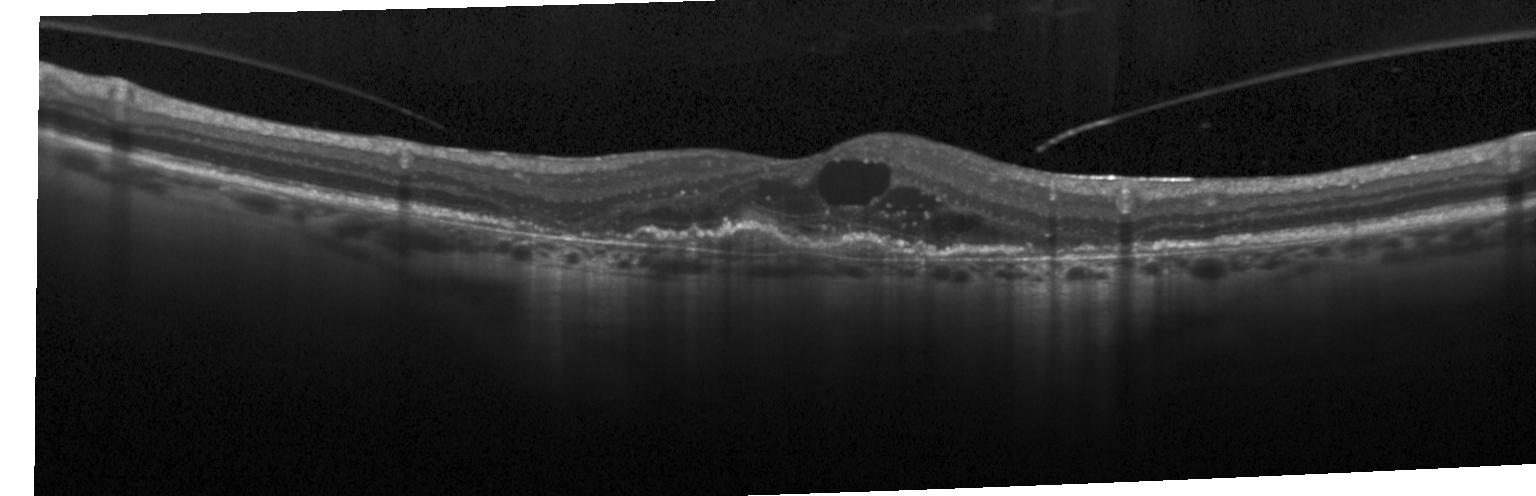

Optical coherence tomography scan, spectral-domain OCT, fovea-centered, instrument: Heidelberg Spectralis.
Impression: a choroidal neovascular membrane.